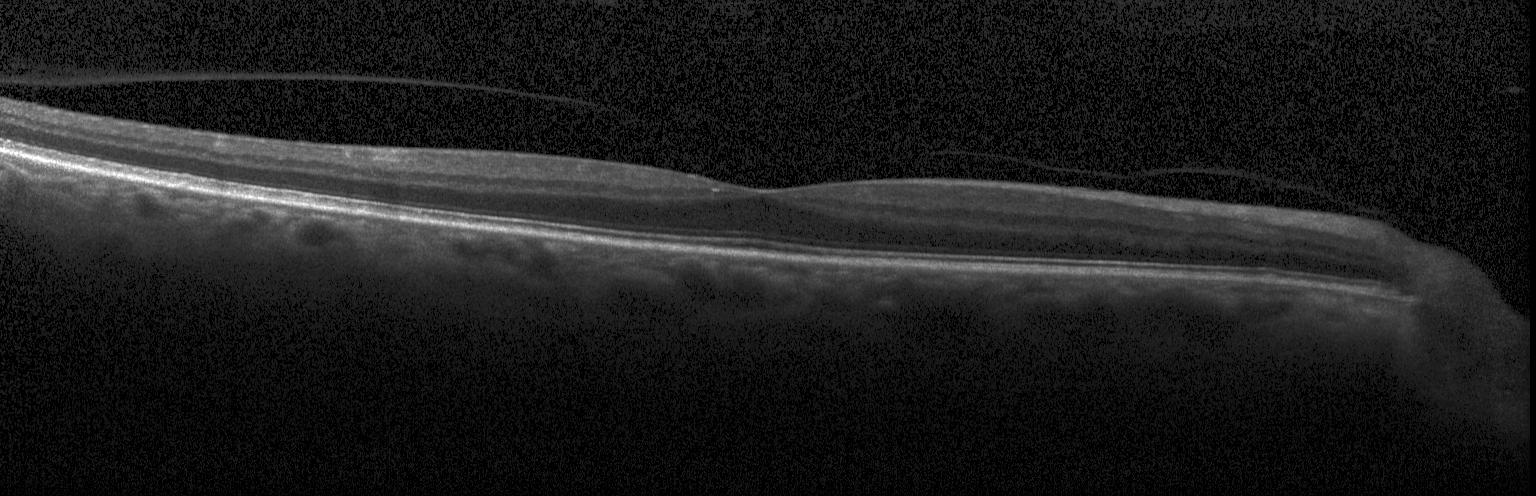 Centered on the fovea; OCT B-scan
Diagnosis: neither choroidal neovascularization, diabetic macular edema, nor drusen.